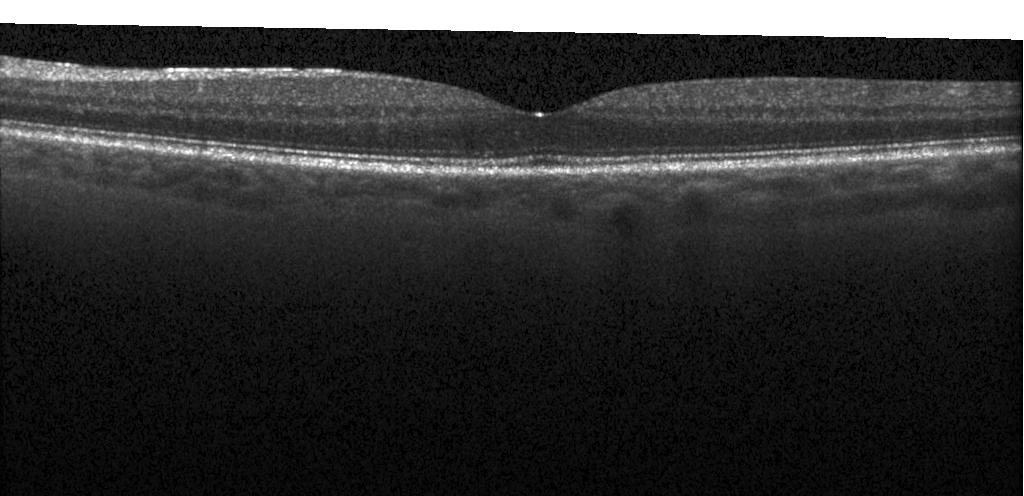 Dx: no choroidal neovascularization, no diabetic macular edema, and no drusen.